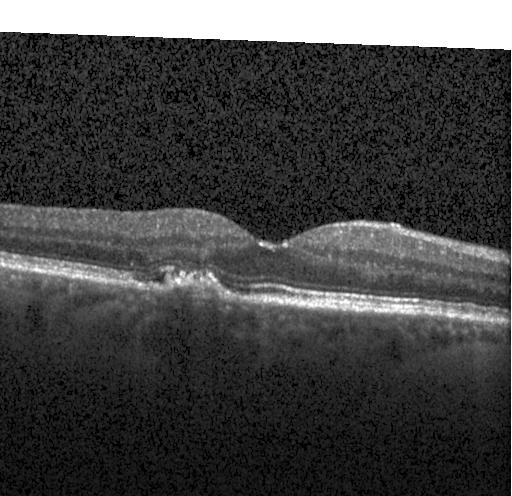 Retinal OCT B-scan
Diagnosis: CNV.